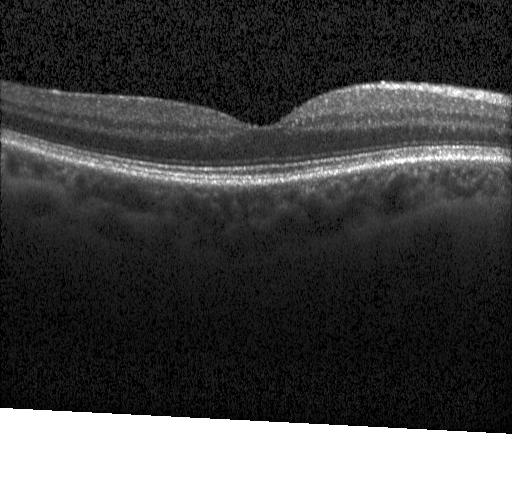 Optical coherence tomography scan. Finding: neither CNV, DME, nor drusen.